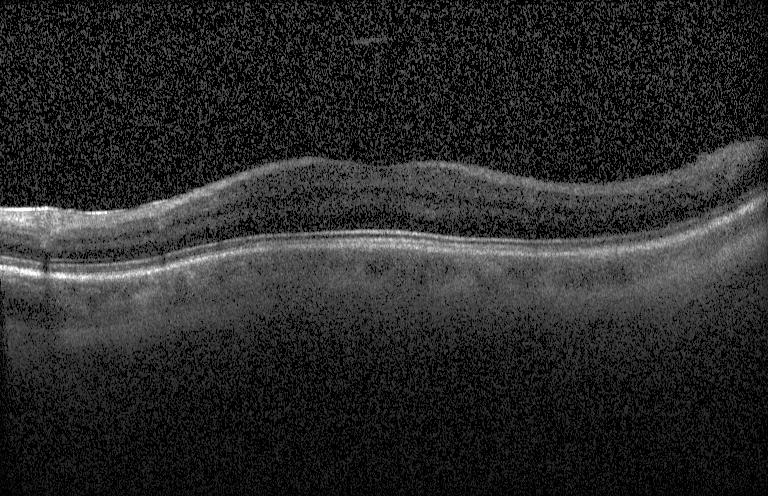

Acquired on a Heidelberg Spectralis, optical coherence tomography scan, spectral-domain optical coherence tomography, horizontal scan through the fovea. Diagnosis: neither choroidal neovascularization, diabetic macular edema, nor drusen.